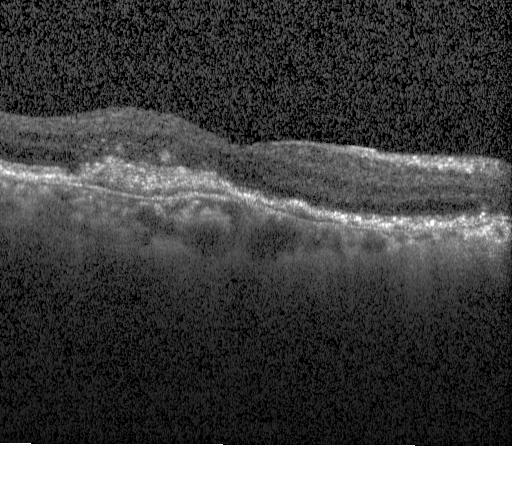 OCT line scan · spectral-domain optical coherence tomography · Heidelberg Spectralis OCT system · fovea-centered — Diagnosis: choroidal neovascularization.